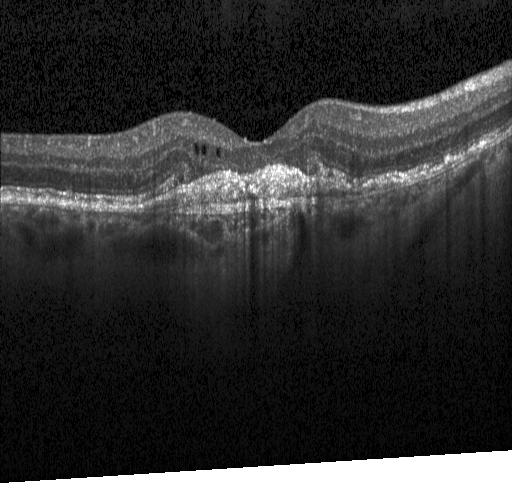

OCT B-scan showing choroidal neovascularization.